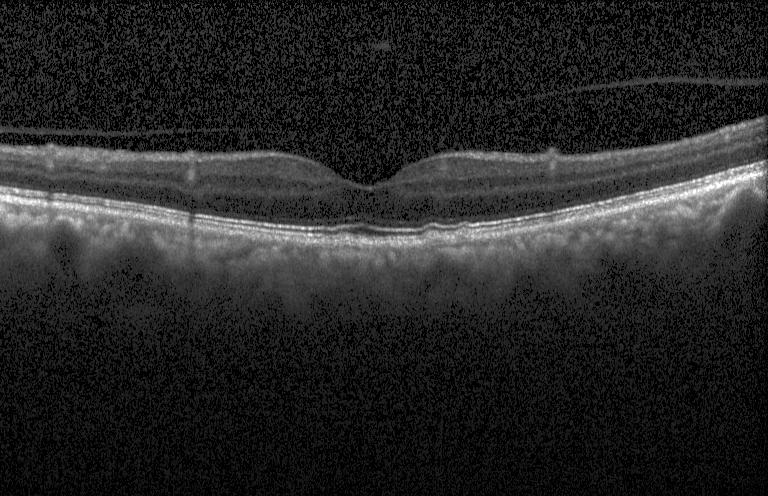 Macular OCT: sub-RPE drusenoid deposits.